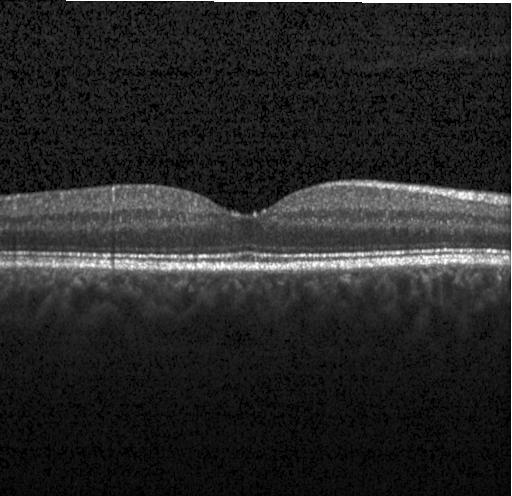

Impression: no choroidal neovascularization, diabetic macular edema, or drusen.